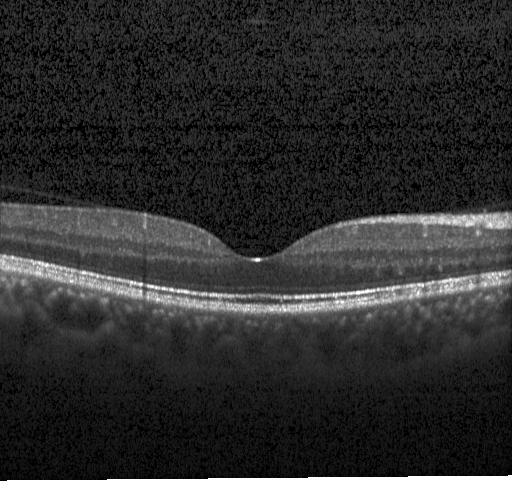 Optical coherence tomography scan; spectral-domain OCT
Macular OCT: no choroidal neovascularization, diabetic macular edema, or drusen.